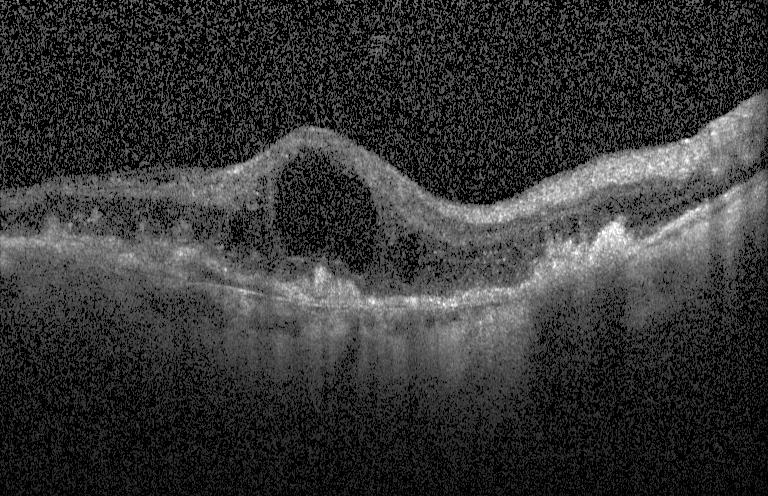 Heidelberg Spectralis. SD-OCT. OCT B-scan. Centered on the fovea — Finding: CNV.